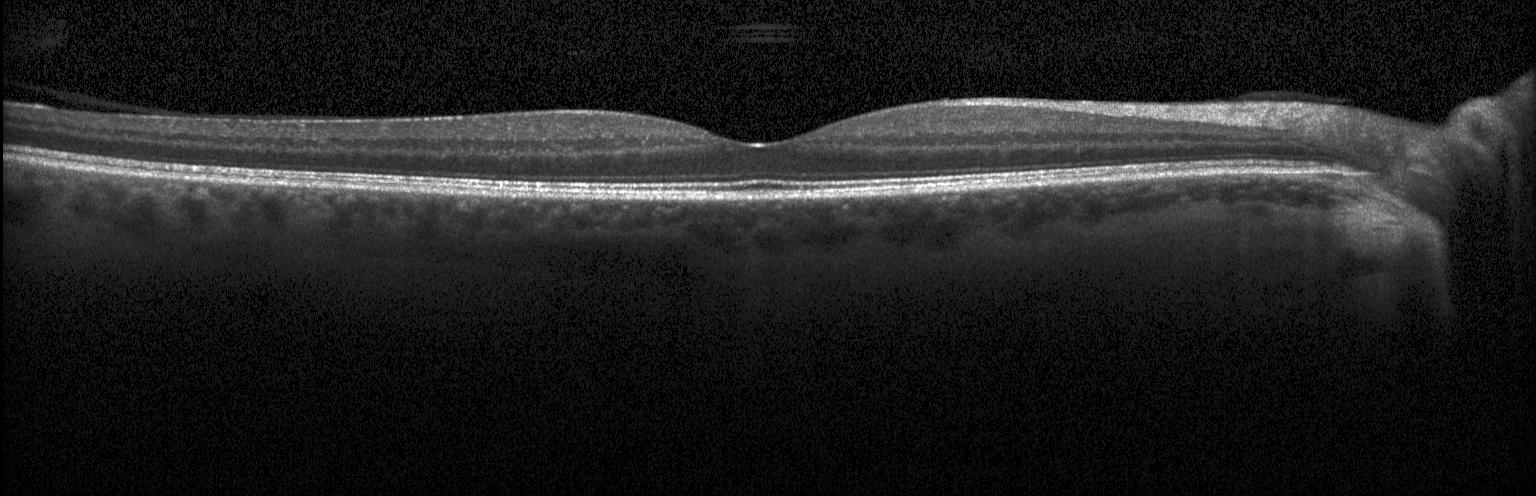 Heidelberg Spectralis. Optical coherence tomography scan. Centered on the fovea.
Diagnosis: no evidence of choroidal neovascularization, diabetic macular edema, or drusen.